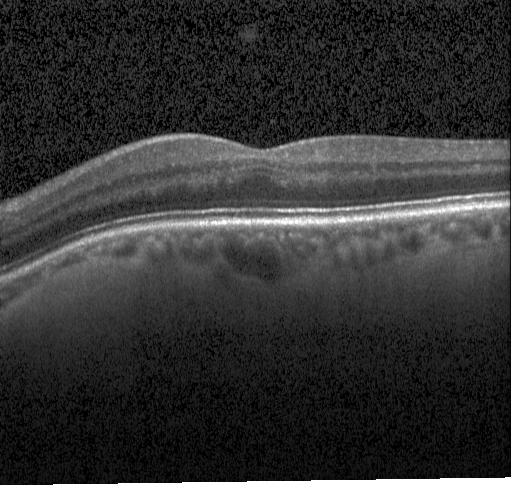 The scan shows no evidence of choroidal neovascularization, diabetic macular edema, or drusen.